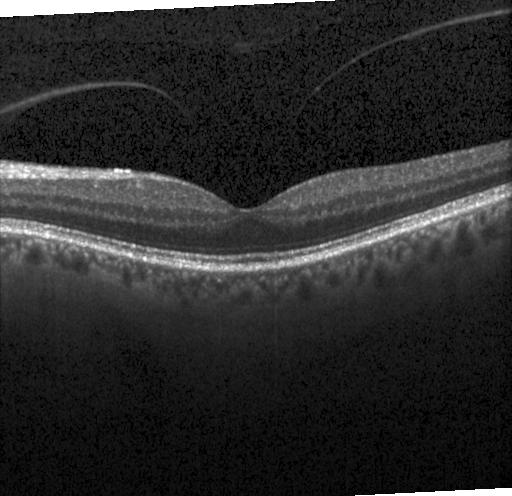
Assessment: no CNV, DME, or drusen.